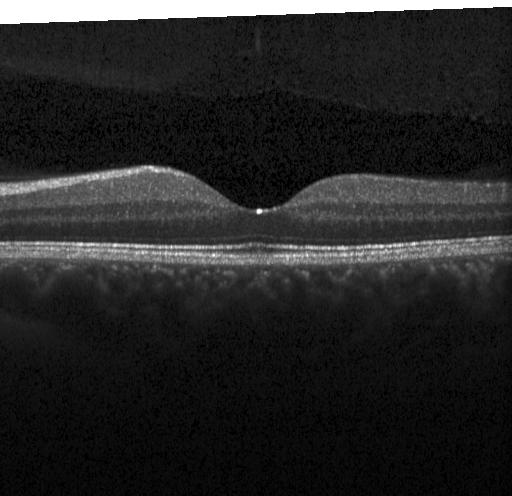
Diagnosis: neither choroidal neovascularization, diabetic macular edema, nor drusen.